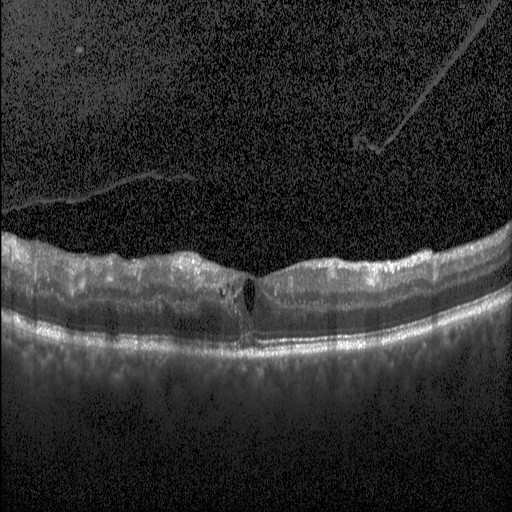

Finding: DME.